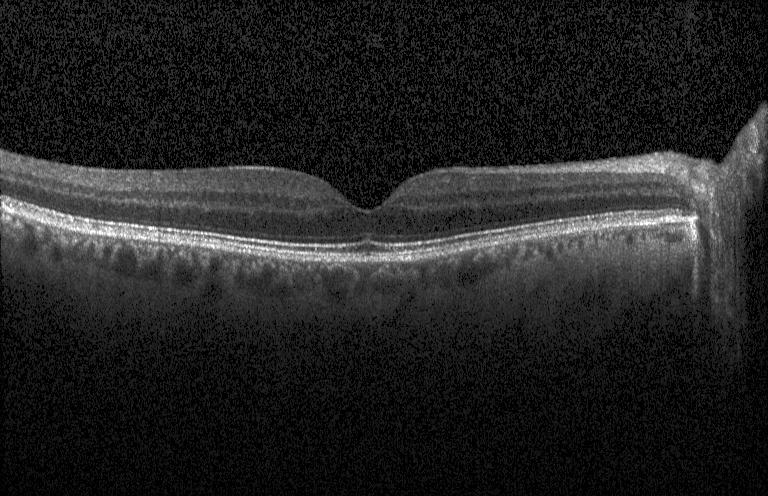 Diagnosis: no choroidal neovascularization, no diabetic macular edema, and no drusen.